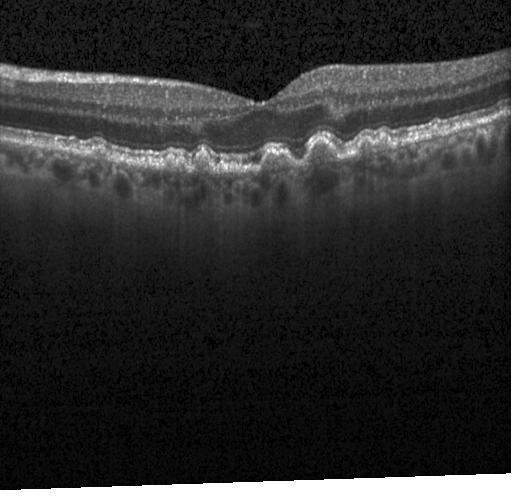
Horizontal scan through the fovea · optical coherence tomography B-scan.
The scan shows drusen.